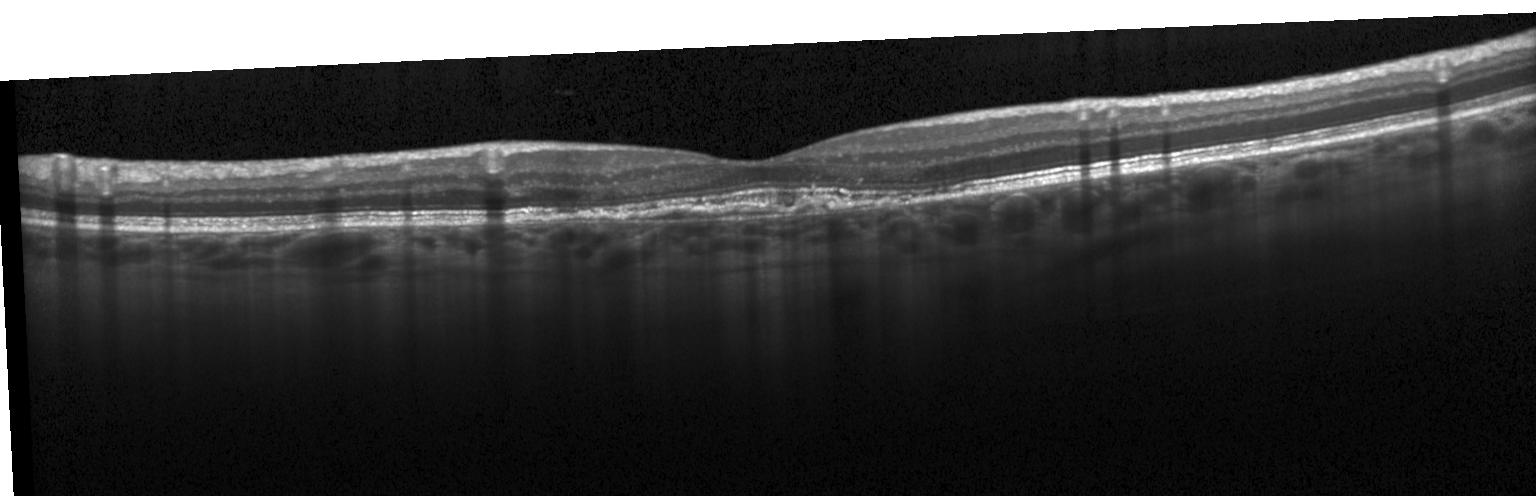

Acquired on a Heidelberg Spectralis; macular scan; retinal OCT B-scan
Dx: CNV.